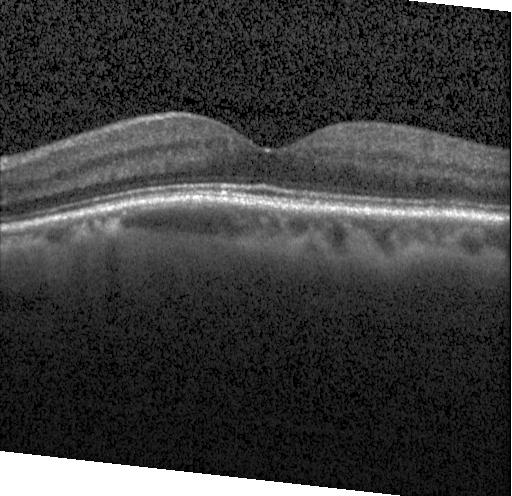
Fovea-centered, SD-OCT, optical coherence tomography scan — Assessment: no choroidal neovascularization, no diabetic macular edema, and no drusen.